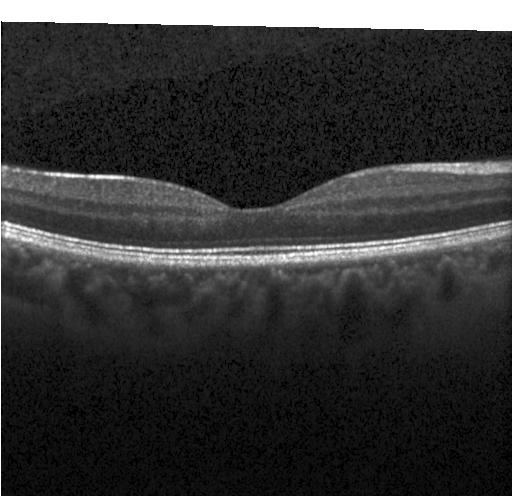
Heidelberg Spectralis OCT system; SD-OCT; retinal OCT B-scan — Diagnosis: no evidence of choroidal neovascularization, diabetic macular edema, or drusen.